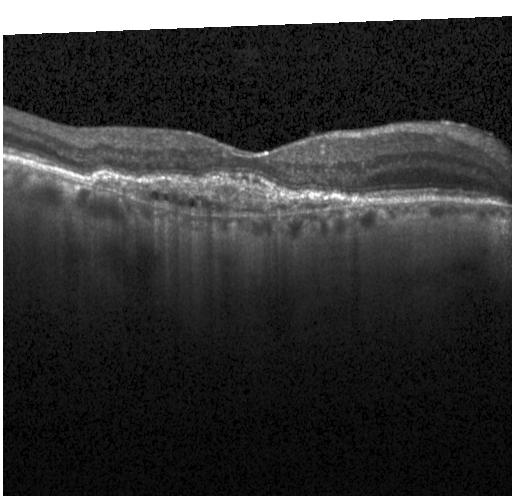

Centered on the fovea, retinal OCT cross-section.
Diagnosis: a choroidal neovascular membrane.